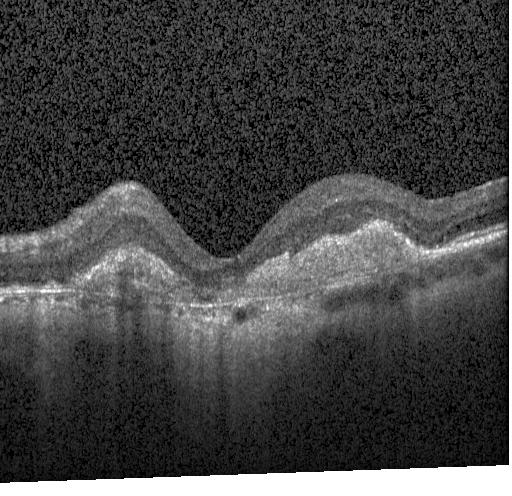

Optical coherence tomography scan; fovea-centered; SD-OCT. Finding: a choroidal neovascular membrane.